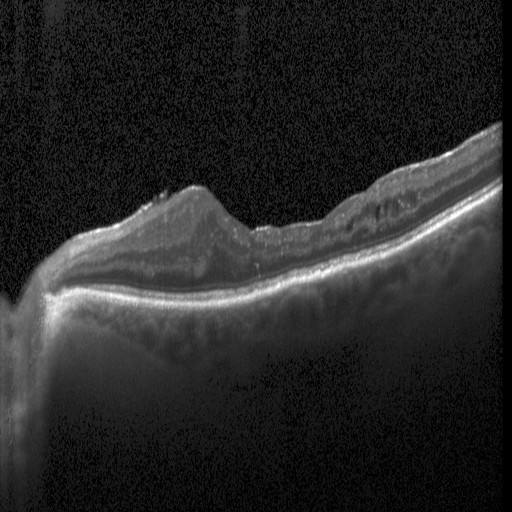

Fovea-centered. SD-OCT. Optical coherence tomography scan.
Macular OCT: DME.